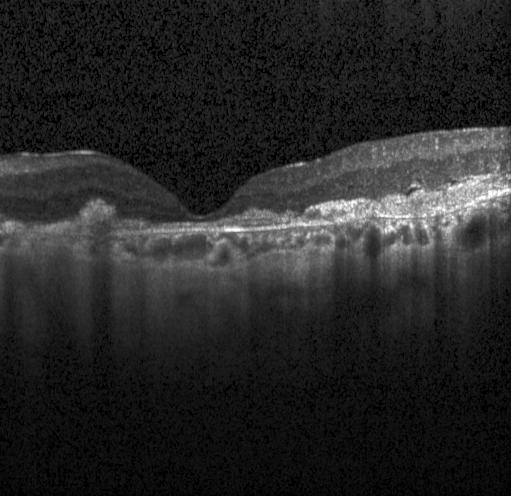

Acquired on a Heidelberg Spectralis. Macular scan. Spectral-domain OCT. Optical coherence tomography B-scan. Assessment: a choroidal neovascular membrane.